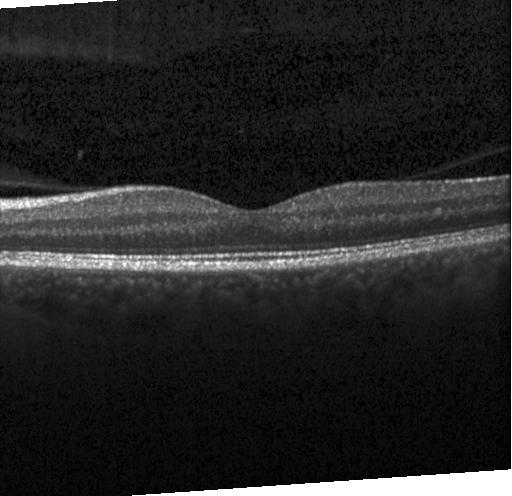

OCT B-scan
No CNV, DME, or drusen.